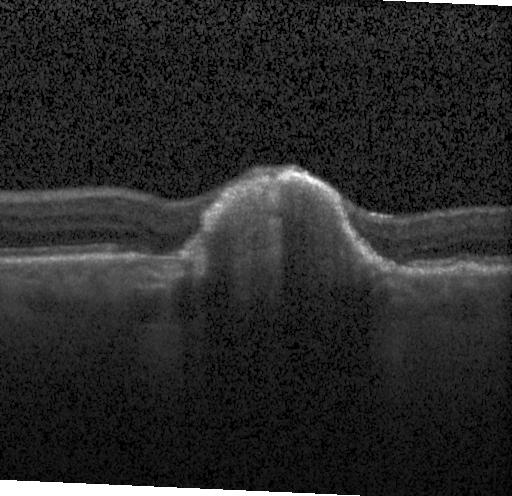
Retinal OCT cross-section; macular scan — Diagnosis: choroidal neovascularization (CNV).